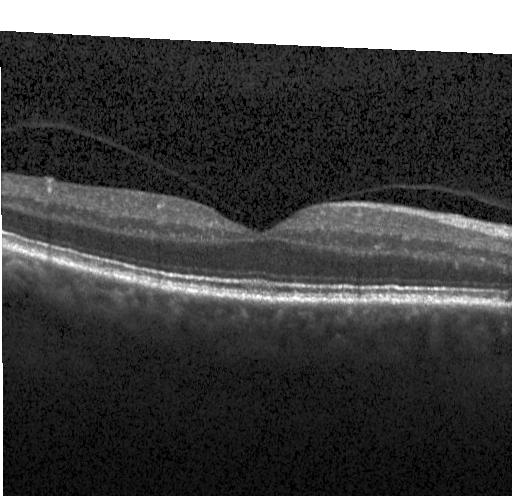 No evidence of CNV, DME, or drusen.